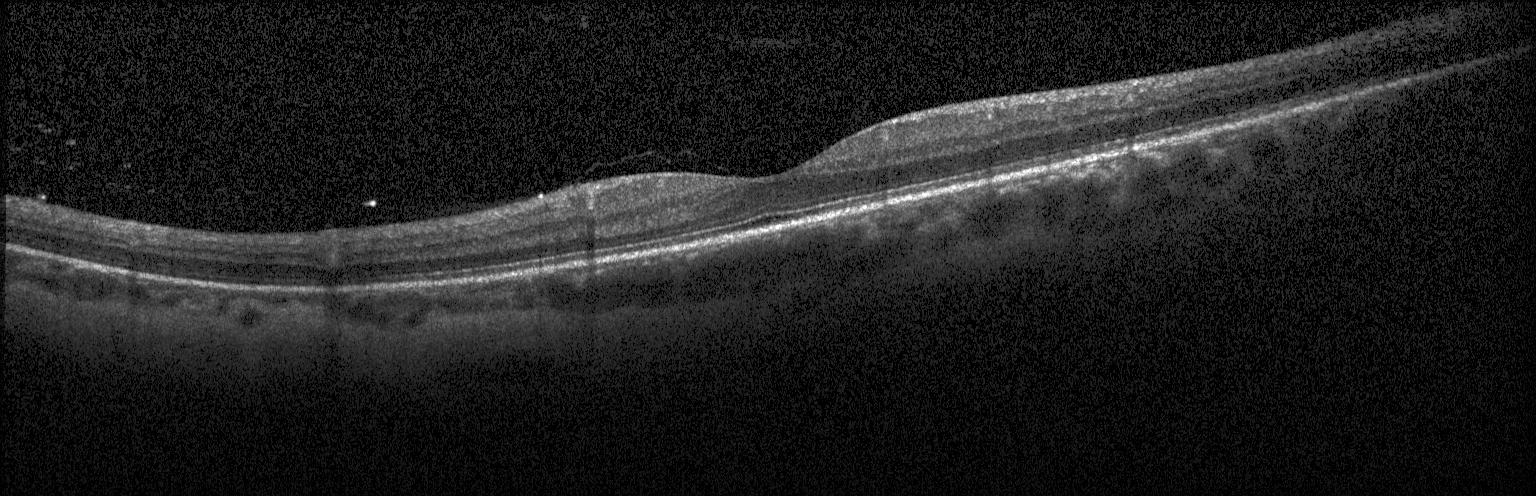

OCT line scan — Finding: no choroidal neovascularization, diabetic macular edema, or drusen.